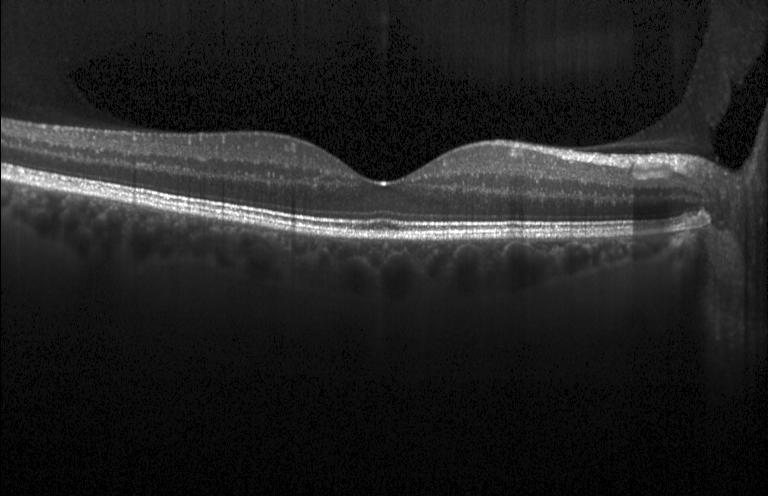 OCT line scan — Assessment: no CNV, DME, or drusen.